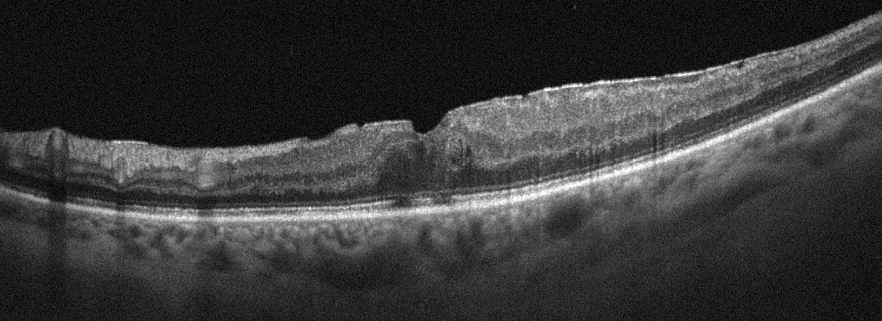
OCT line scan
Assessment: epiretinal membrane.